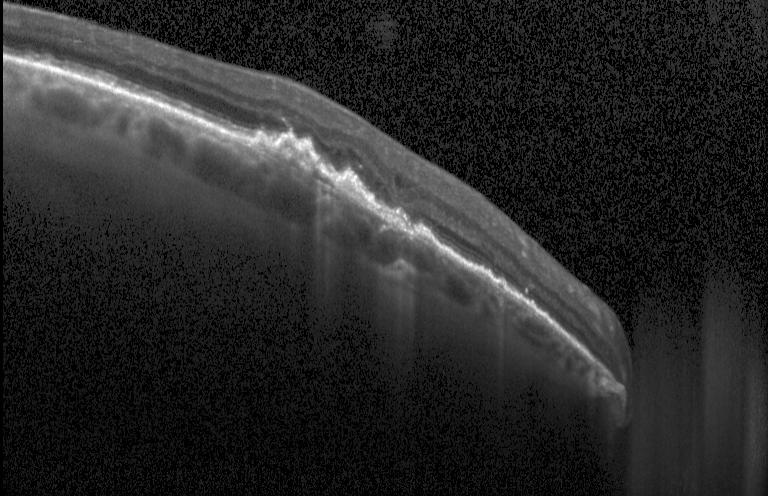
OCT B-scan.
This B-scan demonstrates CNV.